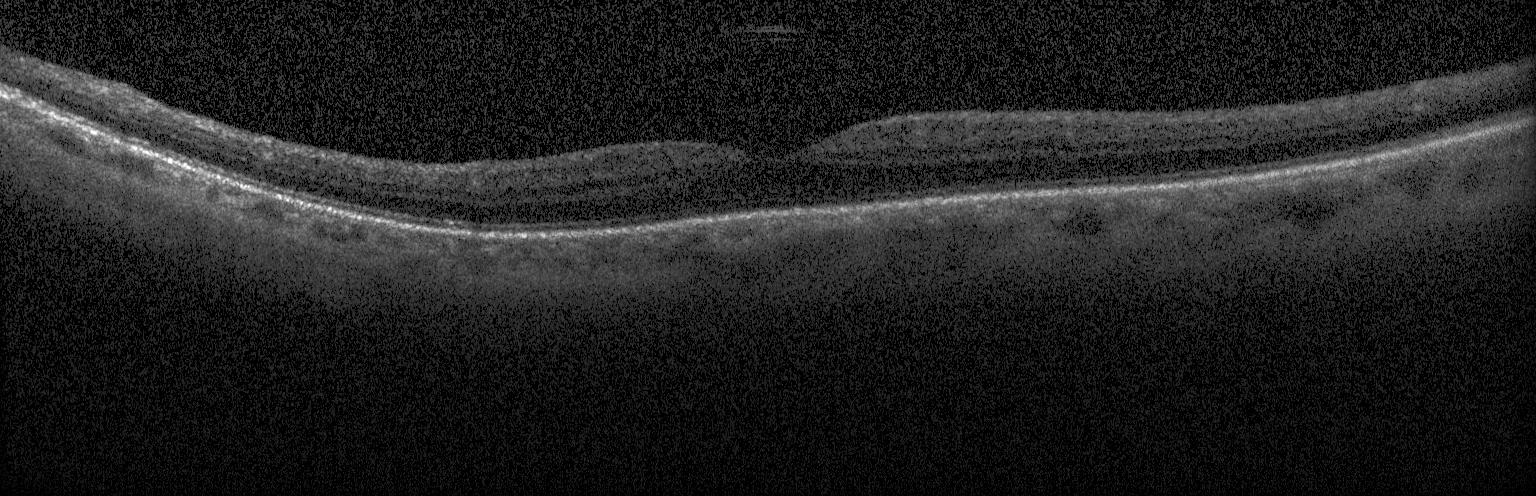
Optical coherence tomography B-scan; through the macula.
Macular OCT: no CNV, no DME, and no drusen.